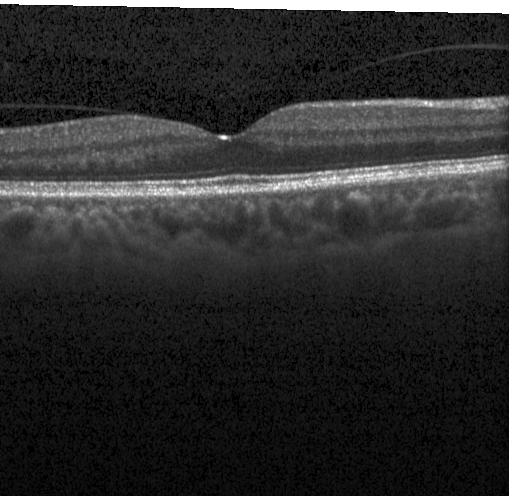

This B-scan demonstrates no evidence of choroidal neovascularization, diabetic macular edema, or drusen.